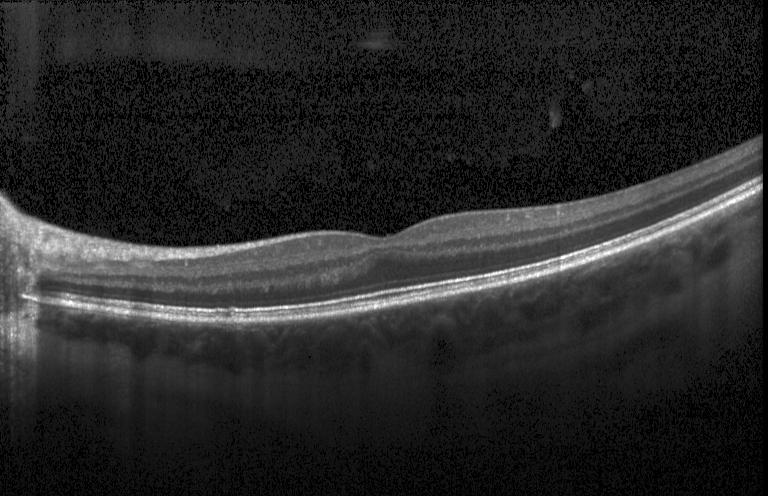
Spectral-domain OCT B-scan: neither CNV, DME, nor drusen.